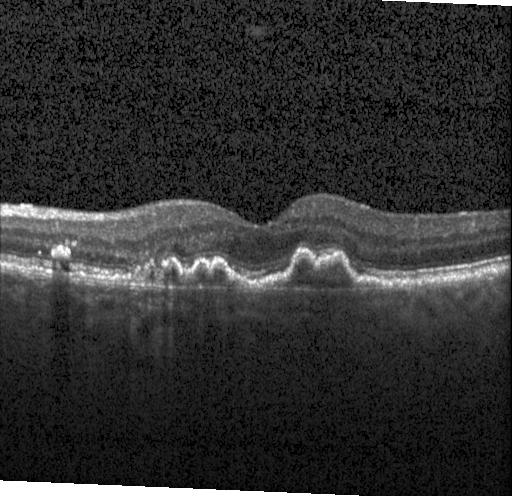
Centered on the fovea; retinal OCT cross-section
A choroidal neovascular membrane.